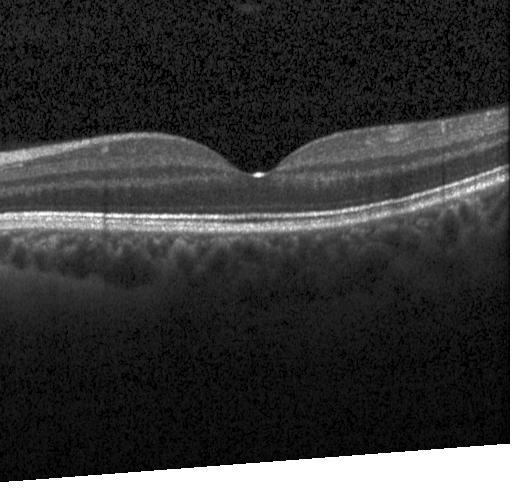
OCT scan showing no evidence of choroidal neovascularization, diabetic macular edema, or drusen.